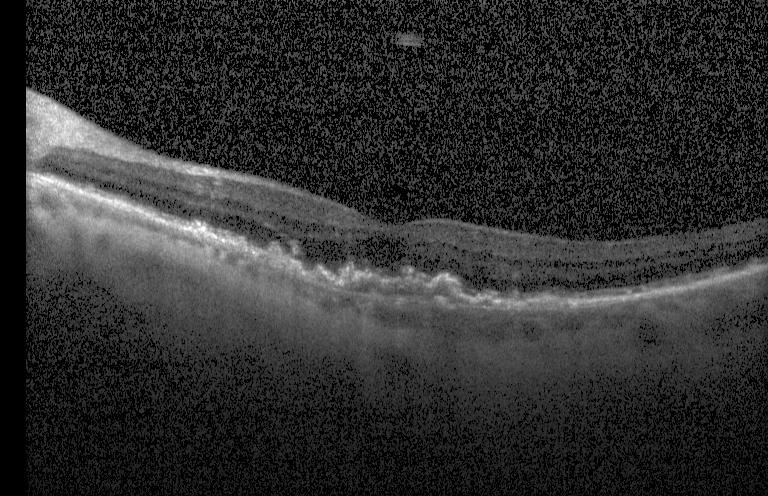
Spectral-domain OCT. OCT line scan. Horizontal scan through the fovea — Finding: choroidal neovascularization (CNV).